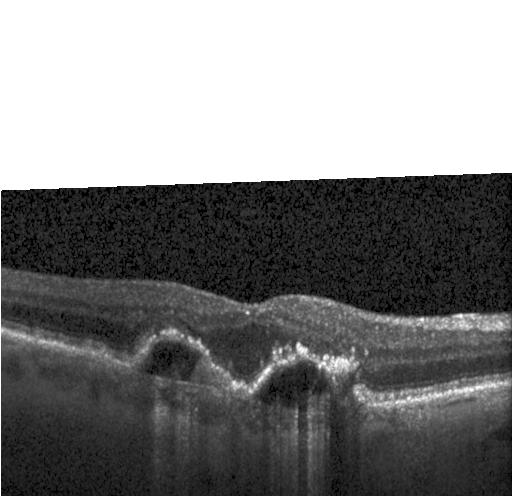 Finding: a choroidal neovascular membrane.